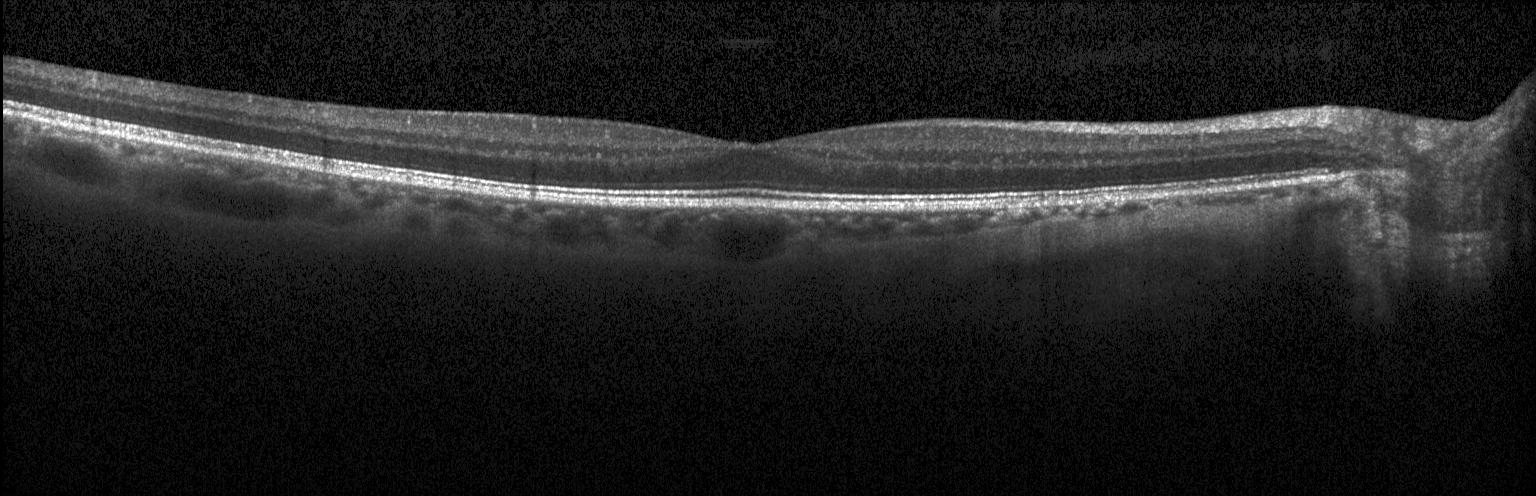
Spectral-domain OCT B-scan: no CNV, DME, or drusen.